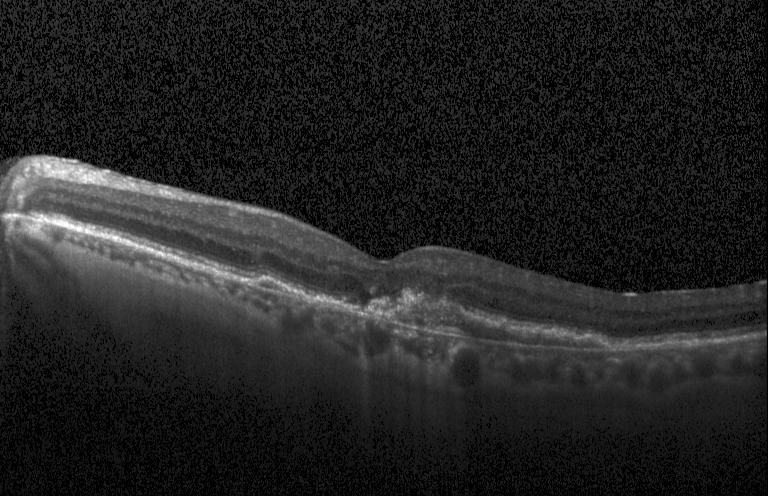

Impression: CNV.